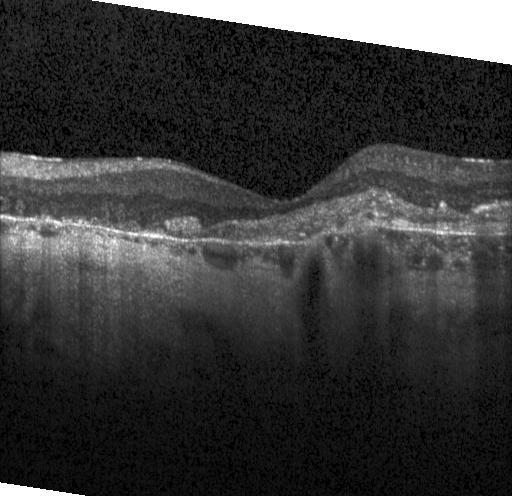

OCT line scan.
Impression: choroidal neovascularization (CNV).